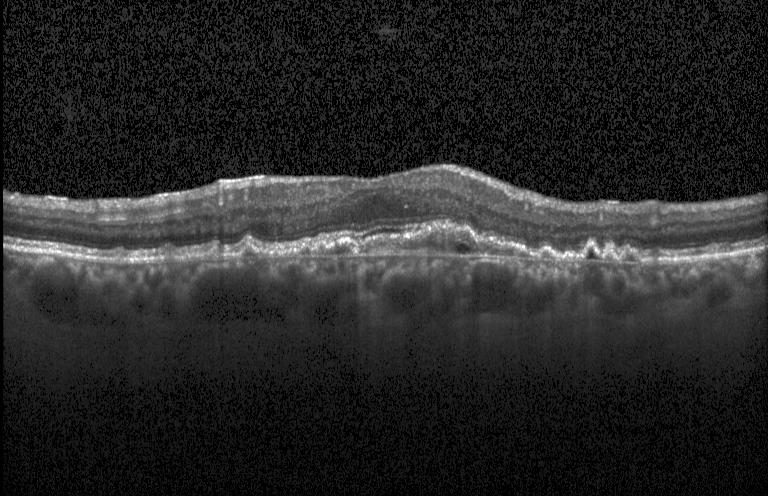 Spectral-domain OCT B-scan: choroidal neovascularization.